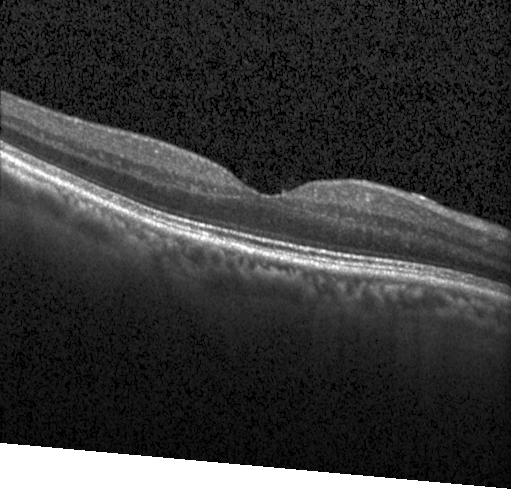

Retinal OCT B-scan, instrument: Heidelberg Spectralis.
Diagnosis: no evidence of CNV, DME, or drusen.